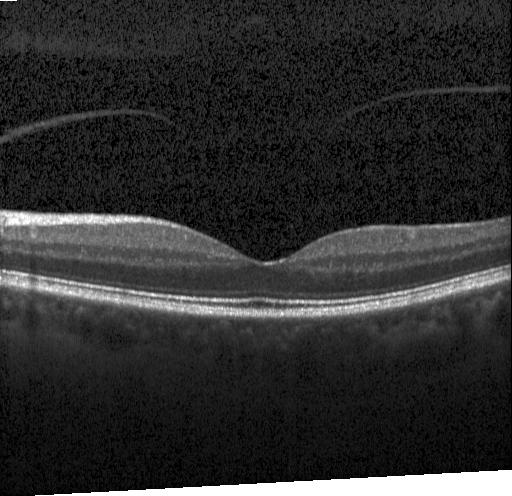
Retinal OCT B-scan.
Dx: neither CNV, DME, nor drusen.